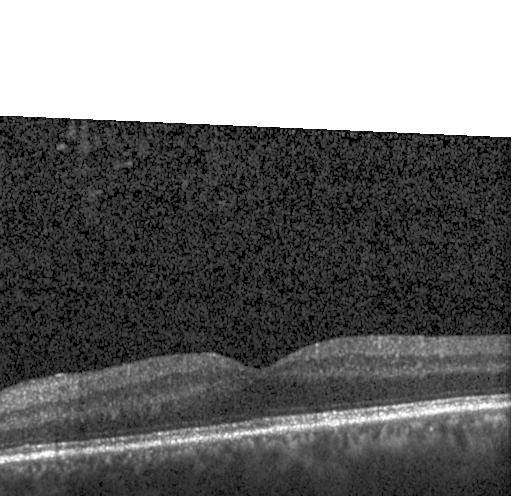

Retinal OCT B-scan · acquired on a Heidelberg Spectralis · spectral-domain OCT. Neither CNV, DME, nor drusen.